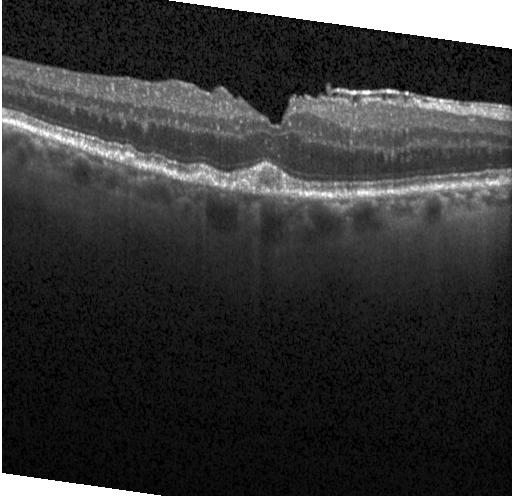

Macular OCT demonstrating multiple drusen.